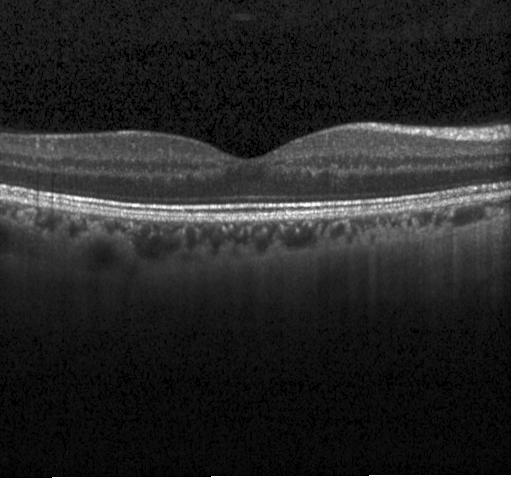

Optical coherence tomography scan — Finding: no evidence of choroidal neovascularization, diabetic macular edema, or drusen.